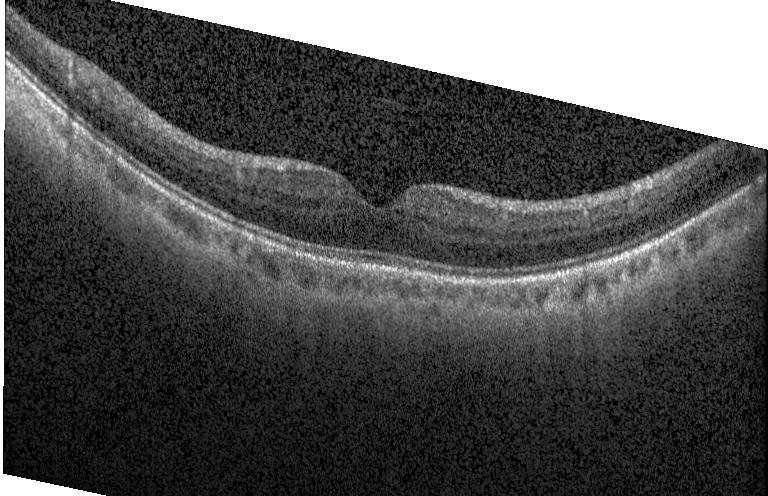 Retinal OCT cross-section showing no choroidal neovascularization, diabetic macular edema, or drusen.